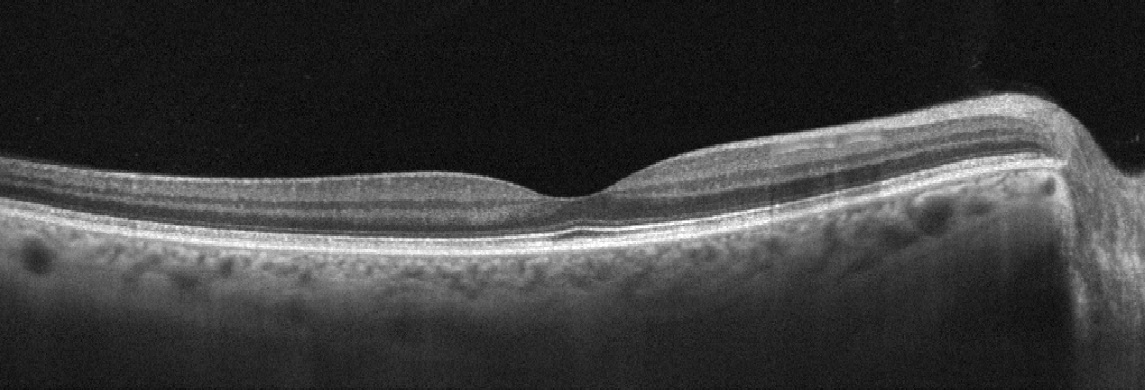 Macular OCT demonstrating no evidence of AMD, DME, ERM, RAO, RVO, or VID.